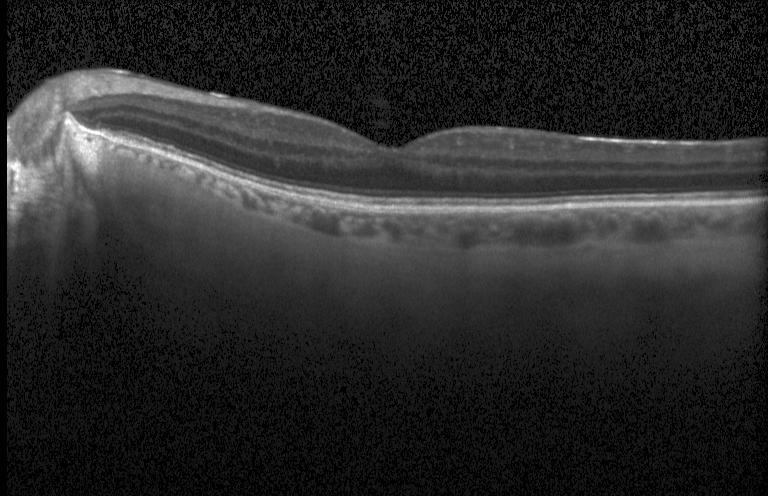 Retinal OCT cross-section showing no choroidal neovascularization, no diabetic macular edema, and no drusen.